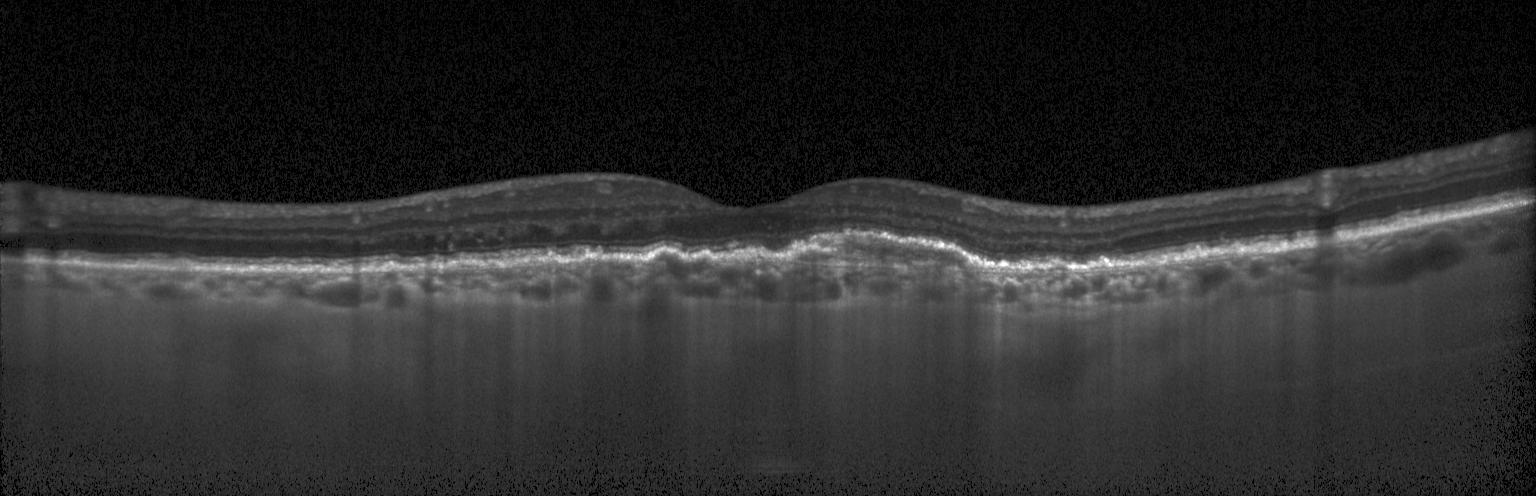

Horizontal scan through the fovea. Retinal OCT B-scan. Heidelberg Spectralis — Impression: choroidal neovascularization (CNV).